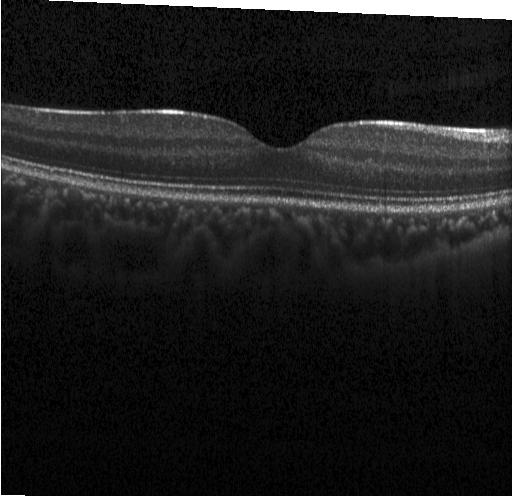 OCT line scan; macular scan; instrument: Heidelberg Spectralis; SD-OCT.
Diagnosis: no choroidal neovascularization, diabetic macular edema, or drusen.